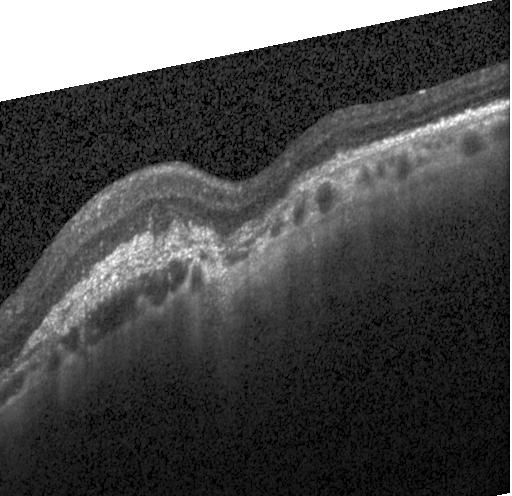
OCT B-scan. A choroidal neovascular membrane.